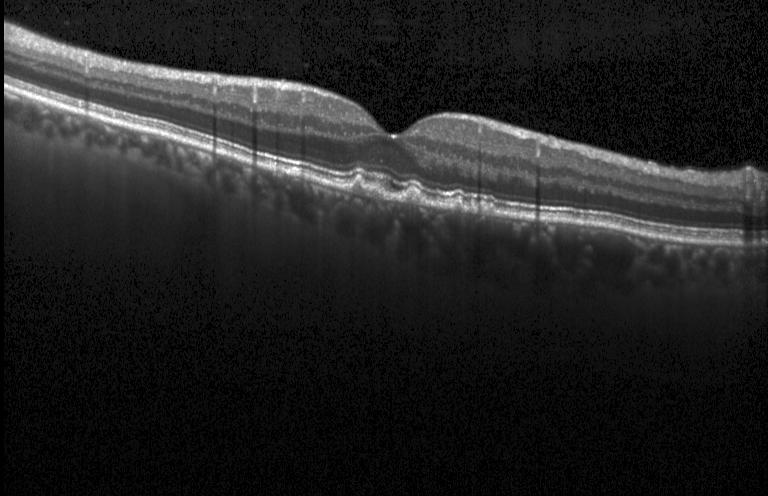 Optical coherence tomography B-scan, spectral-domain optical coherence tomography — Diagnosis: multiple drusen.